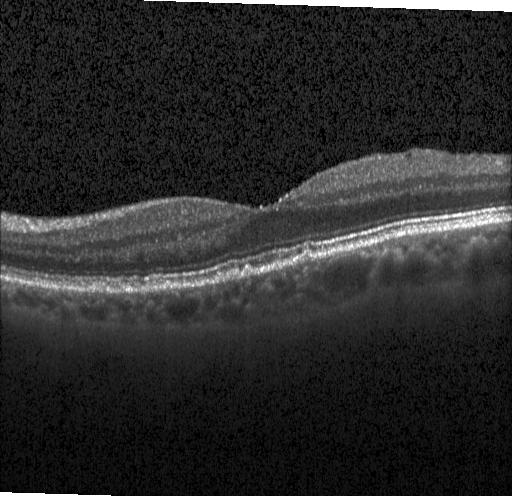 Spectral-domain optical coherence tomography; optical coherence tomography B-scan; instrument: Heidelberg Spectralis. Assessment: multiple drusen.